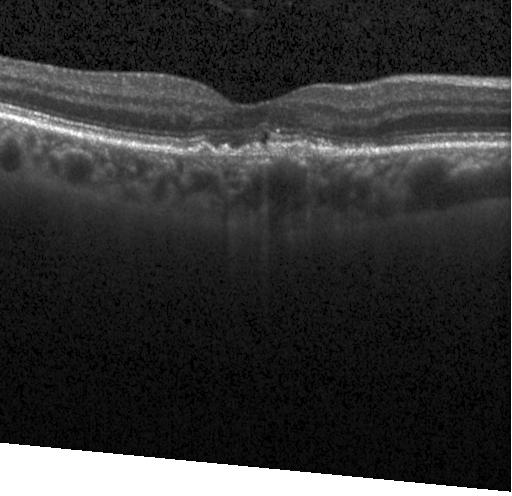

Diagnosis: CNV.